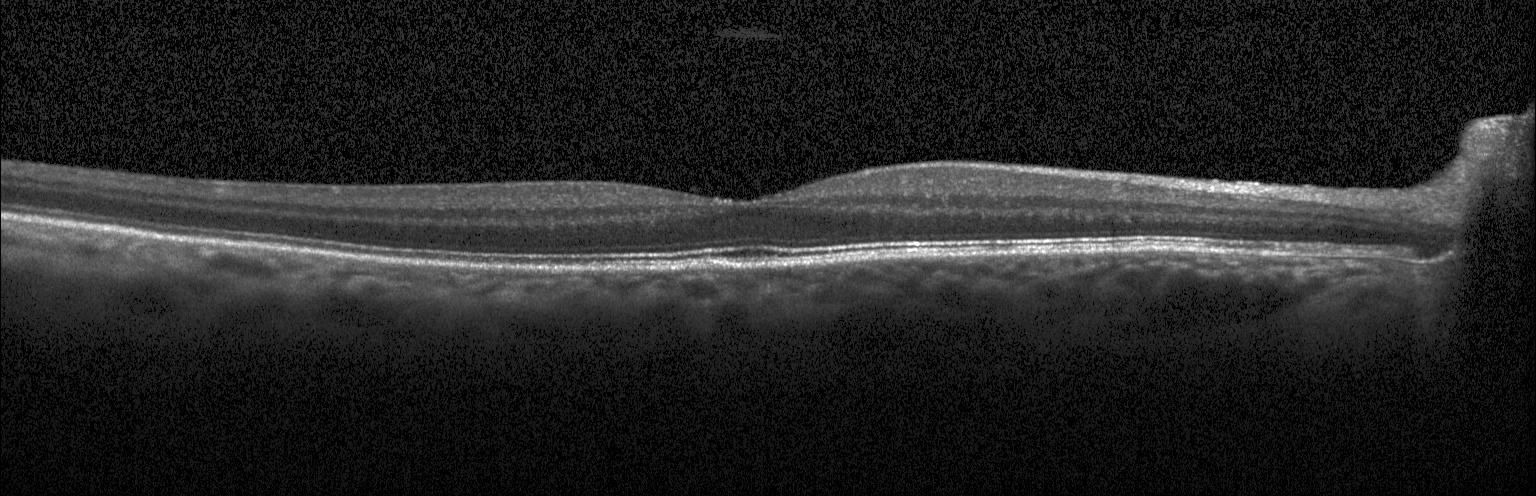 Horizontal scan through the fovea. OCT line scan — Diagnosis: no CNV, DME, or drusen.